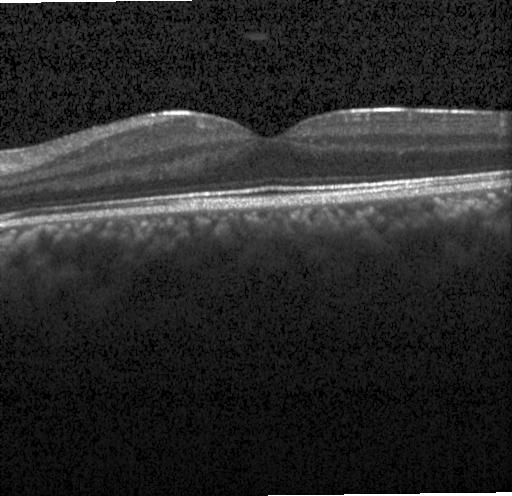
OCT finding: no CNV, DME, or drusen.